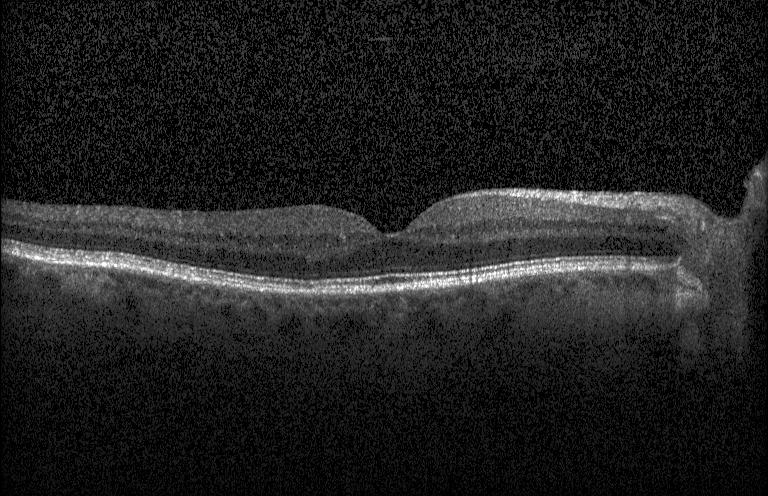
Optical coherence tomography scan
Diagnosis: no evidence of choroidal neovascularization, diabetic macular edema, or drusen.